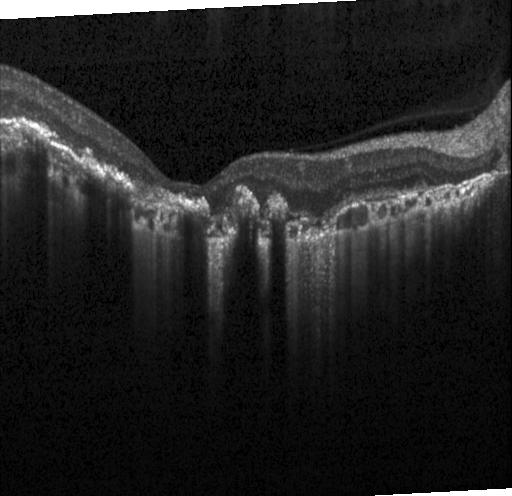
Spectral-domain OCT · retinal OCT cross-section · Heidelberg Spectralis.
Dx: CNV.